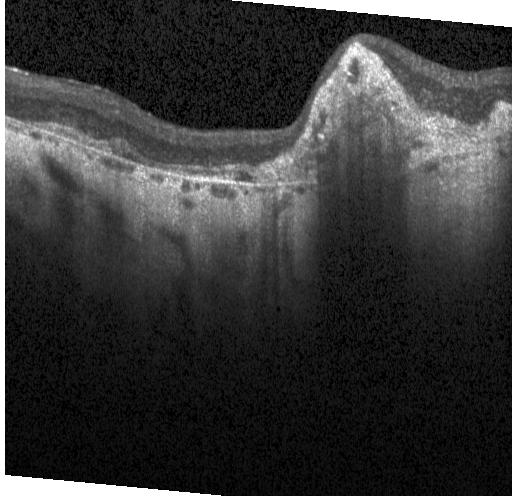
OCT B-scan, horizontal scan through the fovea, spectral-domain OCT, acquired on a Heidelberg Spectralis
Impression: CNV.